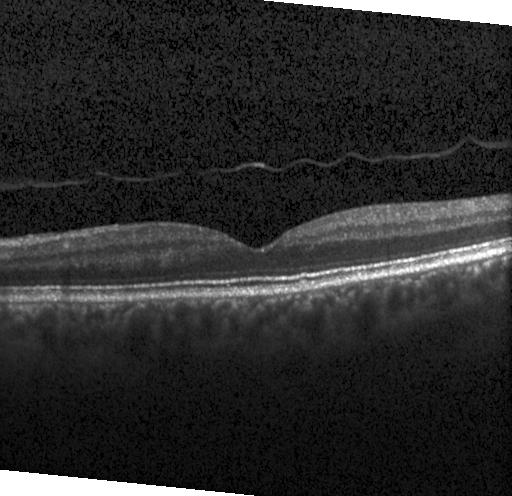
Centered on the fovea; optical coherence tomography B-scan — Assessment: no choroidal neovascularization, no diabetic macular edema, and no drusen.